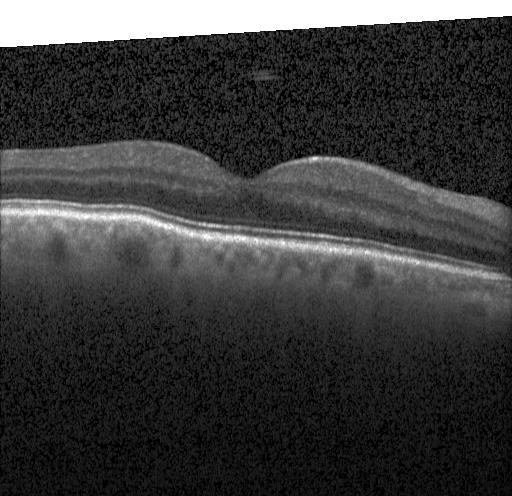 Retinal OCT cross-section showing neither choroidal neovascularization, diabetic macular edema, nor drusen.